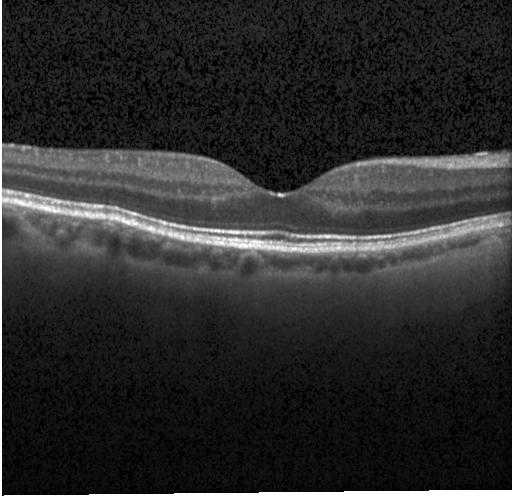

OCT line scan. Instrument: Heidelberg Spectralis. Spectral-domain optical coherence tomography. Dx: no CNV, no DME, and no drusen.